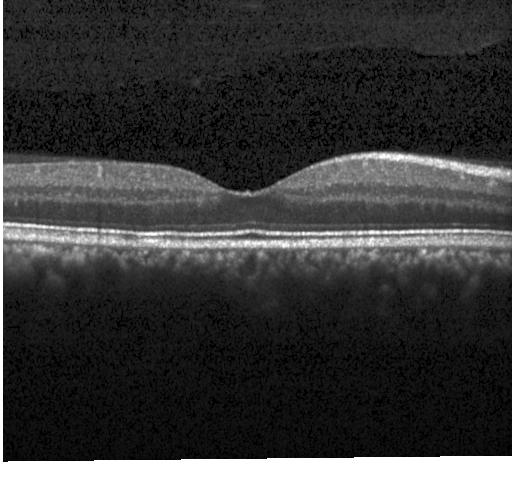

Finding: neither CNV, DME, nor drusen.